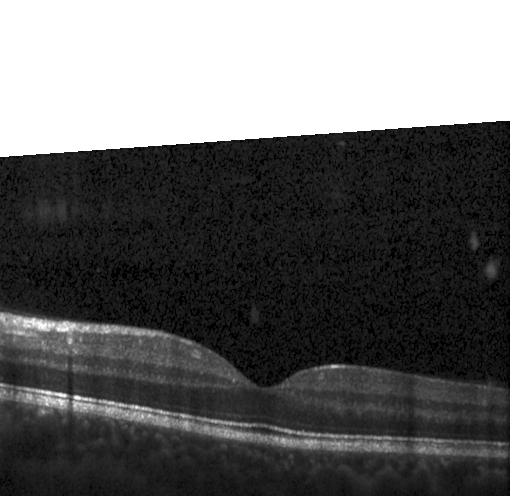
OCT B-scan showing neither choroidal neovascularization, diabetic macular edema, nor drusen.